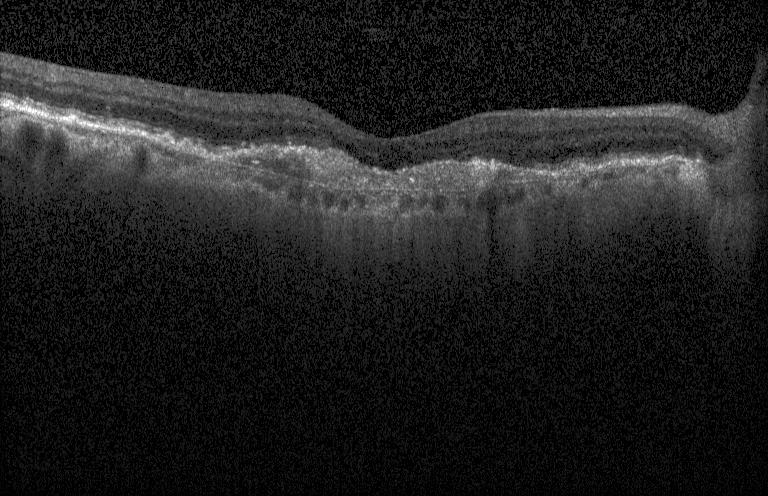

Diagnosis: a choroidal neovascular membrane.